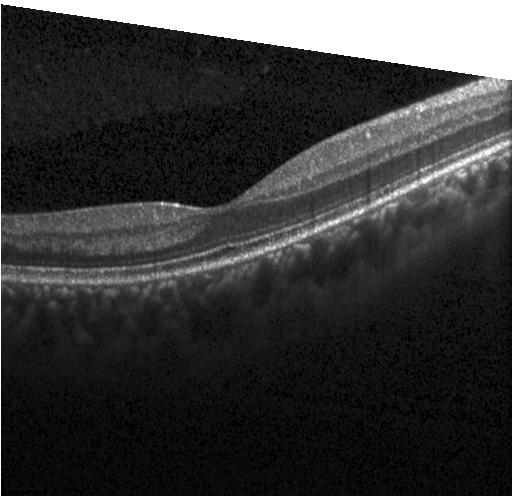
This B-scan demonstrates no evidence of choroidal neovascularization, diabetic macular edema, or drusen.